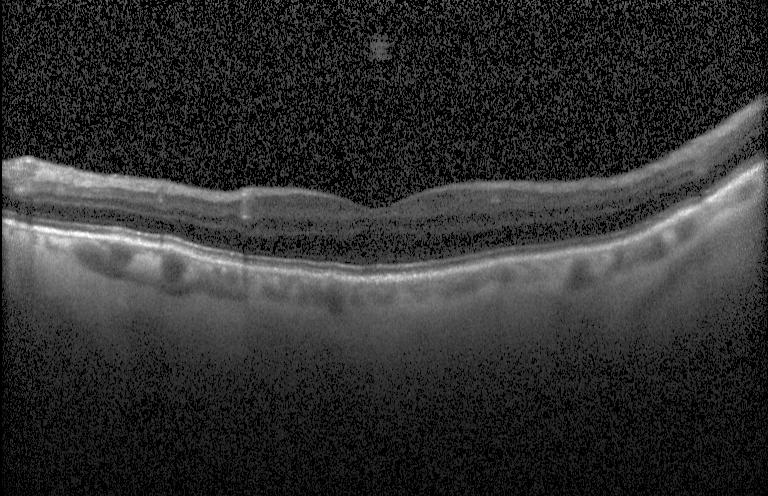 OCT finding: neither choroidal neovascularization, diabetic macular edema, nor drusen.